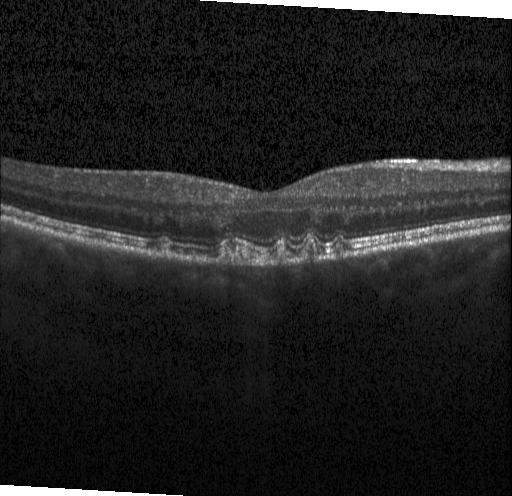
Optical coherence tomography B-scan; horizontal scan through the fovea; acquired on a Heidelberg Spectralis; SD-OCT. Dx: sub-RPE drusenoid deposits.